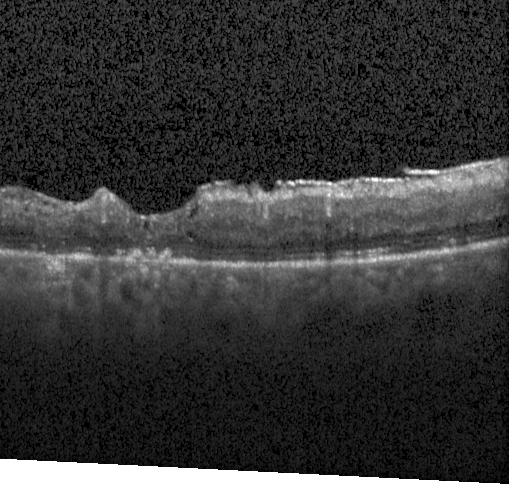
Heidelberg Spectralis, SD-OCT, OCT B-scan, horizontal scan through the fovea. Assessment: CNV.